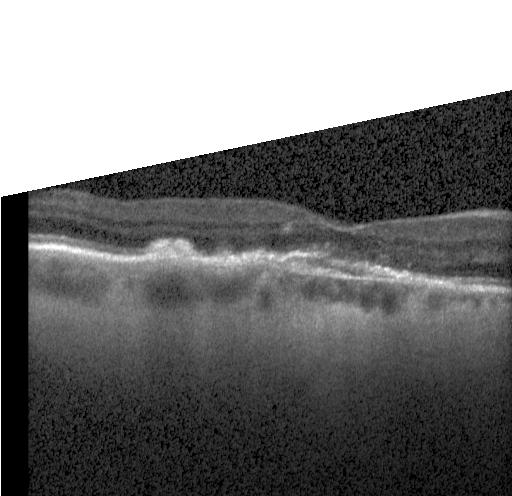 Spectral-domain OCT B-scan: choroidal neovascularization (CNV).